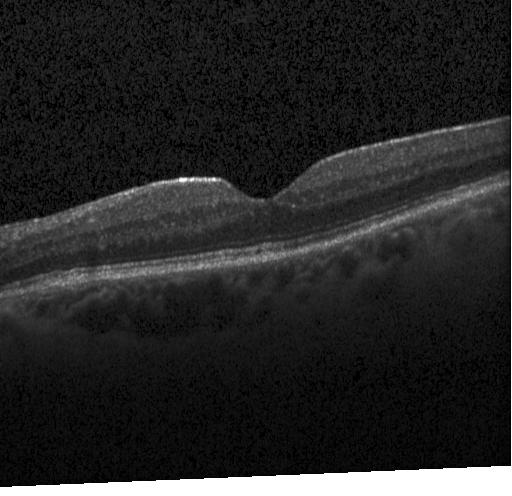
OCT scan showing no evidence of choroidal neovascularization, diabetic macular edema, or drusen.